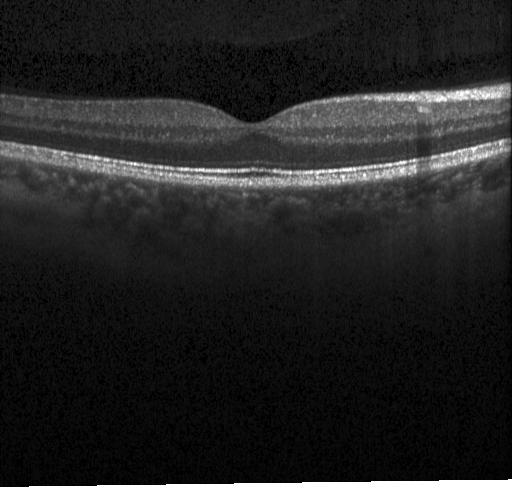

Instrument: Heidelberg Spectralis · through the macula · spectral-domain OCT · optical coherence tomography scan.
The scan shows no CNV, DME, or drusen.